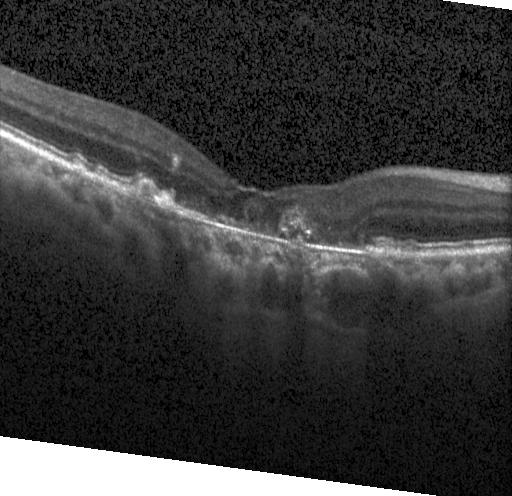

Dx: CNV.